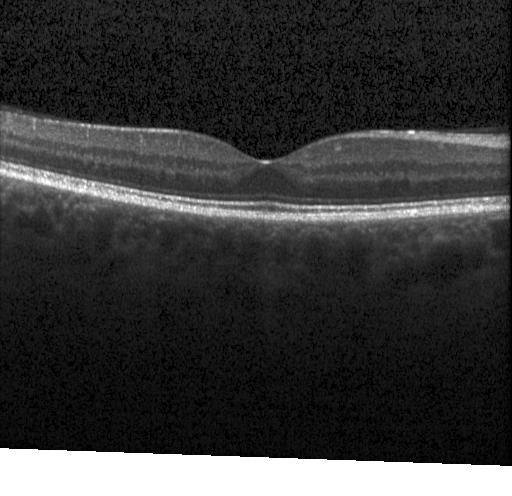
Retinal OCT B-scan · spectral-domain optical coherence tomography
OCT finding: no evidence of choroidal neovascularization, diabetic macular edema, or drusen.